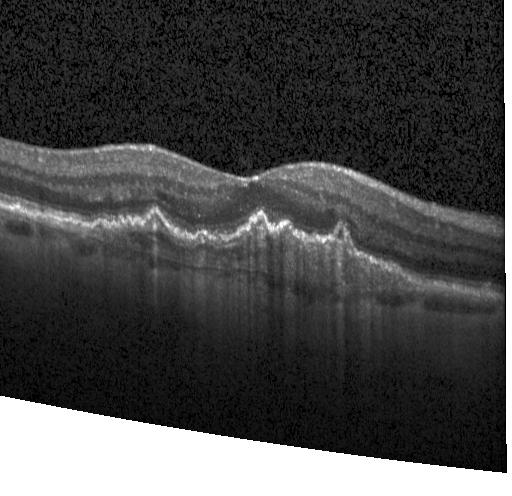
OCT line scan; spectral-domain optical coherence tomography; centered on the fovea; acquired on a Heidelberg Spectralis
This B-scan demonstrates a choroidal neovascular membrane.